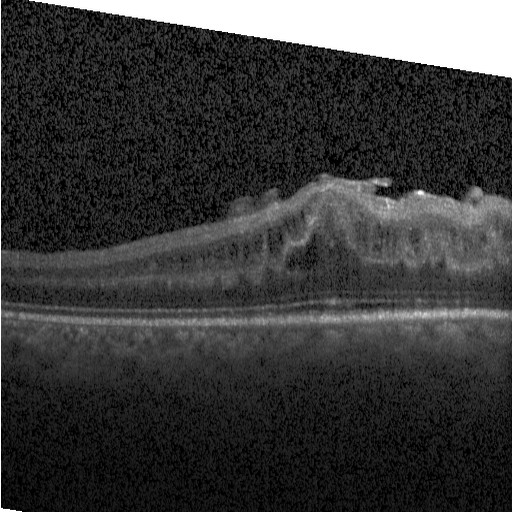

Spectral-domain optical coherence tomography · optical coherence tomography B-scan · Heidelberg Spectralis OCT system. This B-scan demonstrates DME.